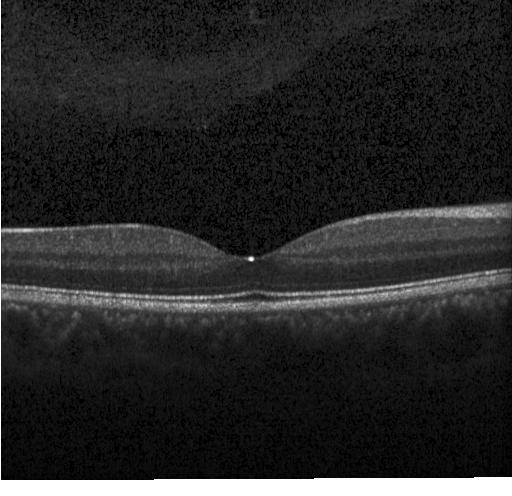

Retinal OCT cross-section showing no choroidal neovascularization, no diabetic macular edema, and no drusen.